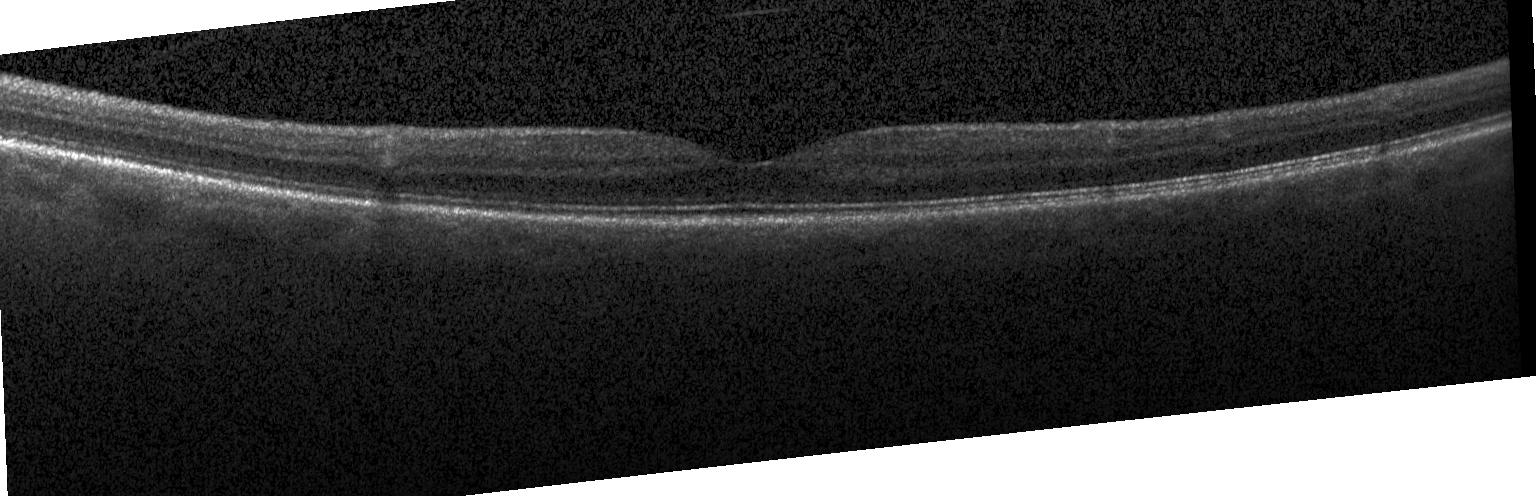 Macular OCT: no choroidal neovascularization, diabetic macular edema, or drusen.